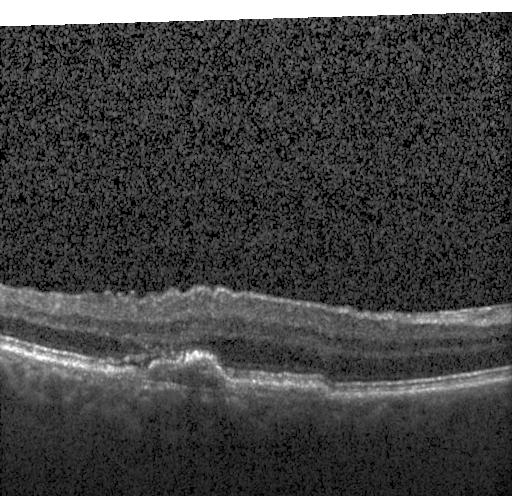 Fovea-centered; OCT line scan — Diagnosis: CNV.